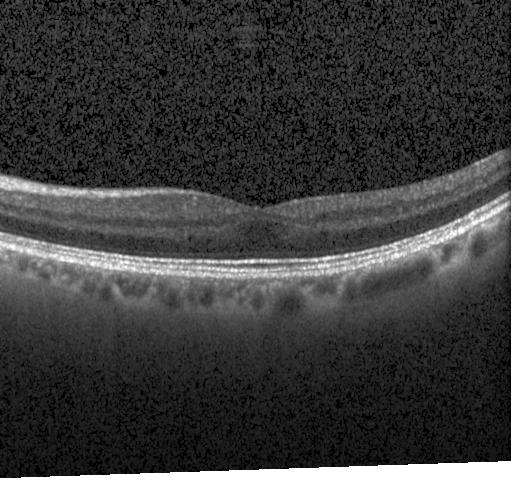
OCT B-scan; acquired on a Heidelberg Spectralis; spectral-domain optical coherence tomography; horizontal scan through the fovea — Impression: no choroidal neovascularization, no diabetic macular edema, and no drusen.